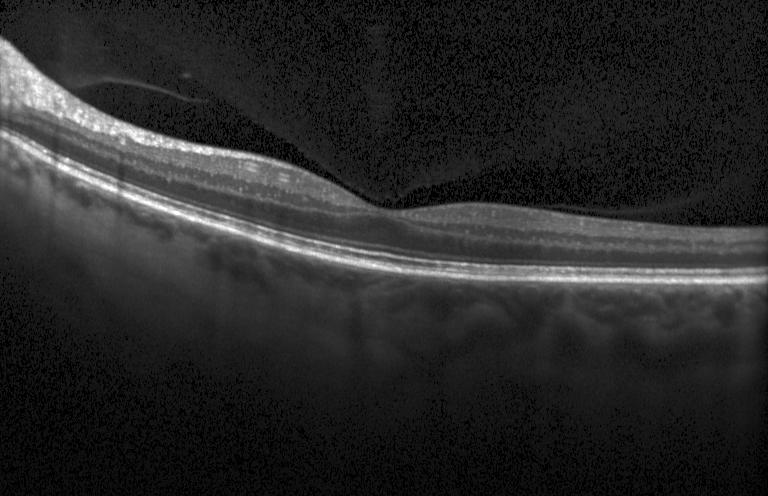 Optical coherence tomography scan — Dx: no CNV, no DME, and no drusen.